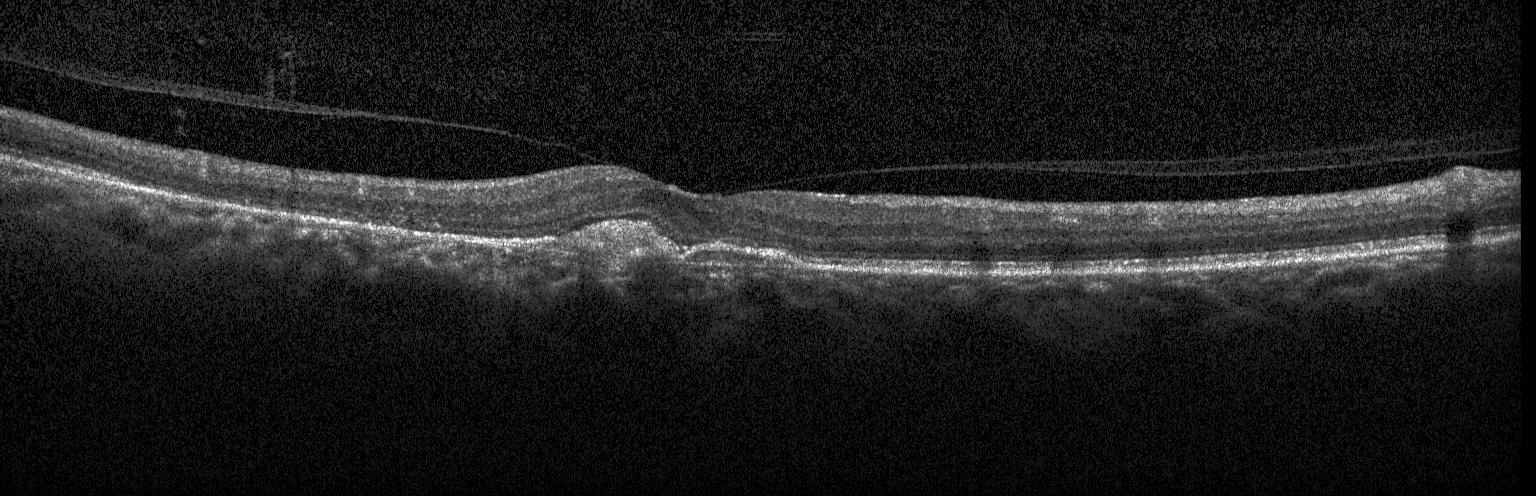 Fovea-centered, spectral-domain optical coherence tomography, Heidelberg Spectralis, OCT B-scan.
Finding: a choroidal neovascular membrane.